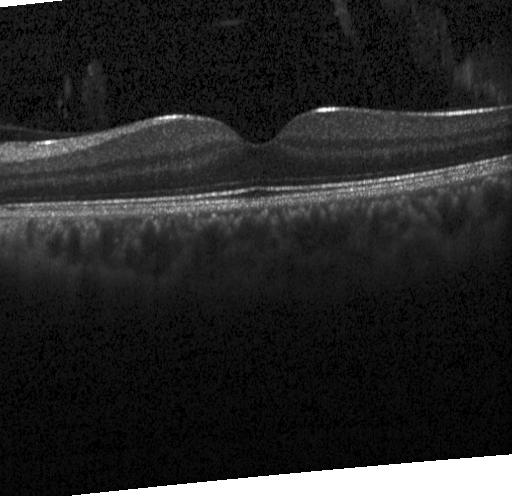
Heidelberg Spectralis OCT system; through the macula; optical coherence tomography B-scan; spectral-domain optical coherence tomography. Dx: no evidence of CNV, DME, or drusen.